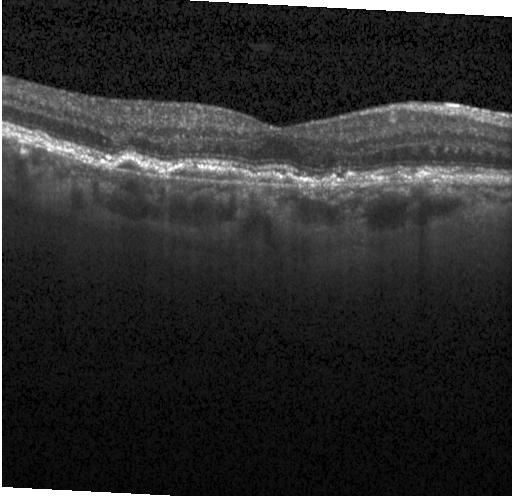

This B-scan demonstrates CNV.